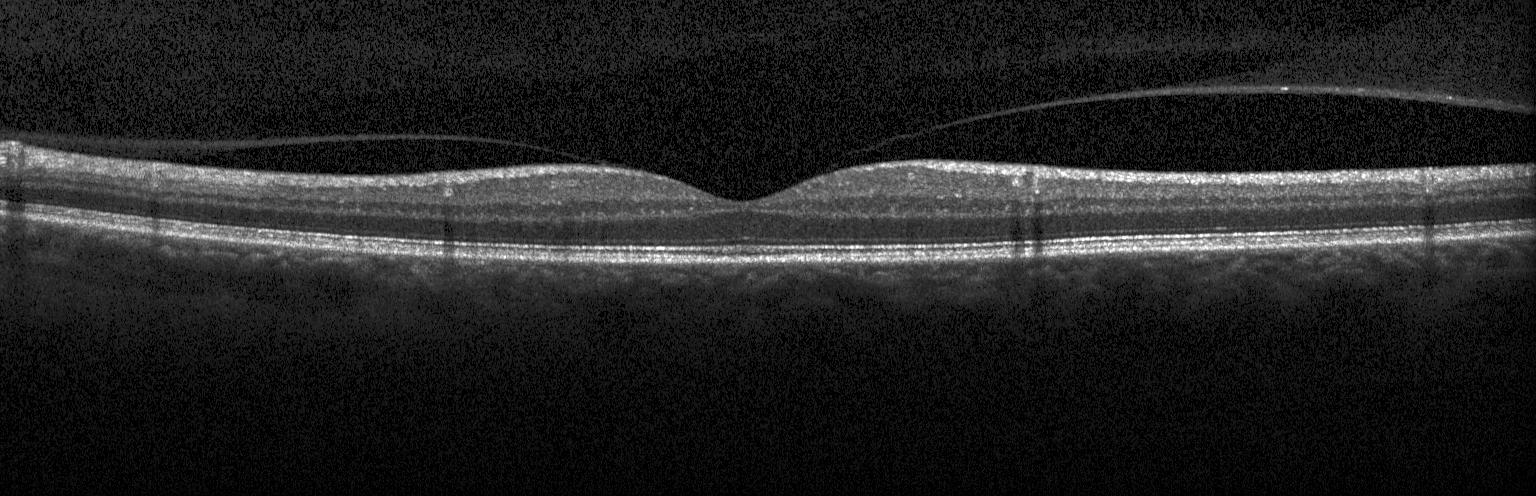
Retinal OCT cross-section; spectral-domain OCT
Finding: no CNV, no DME, and no drusen.